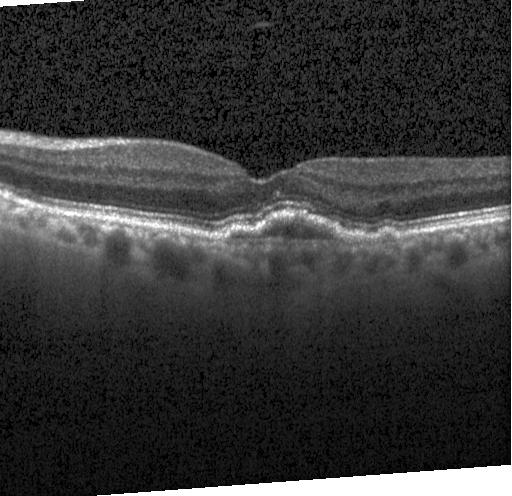 Spectral-domain OCT · OCT line scan
Finding: a choroidal neovascular membrane.